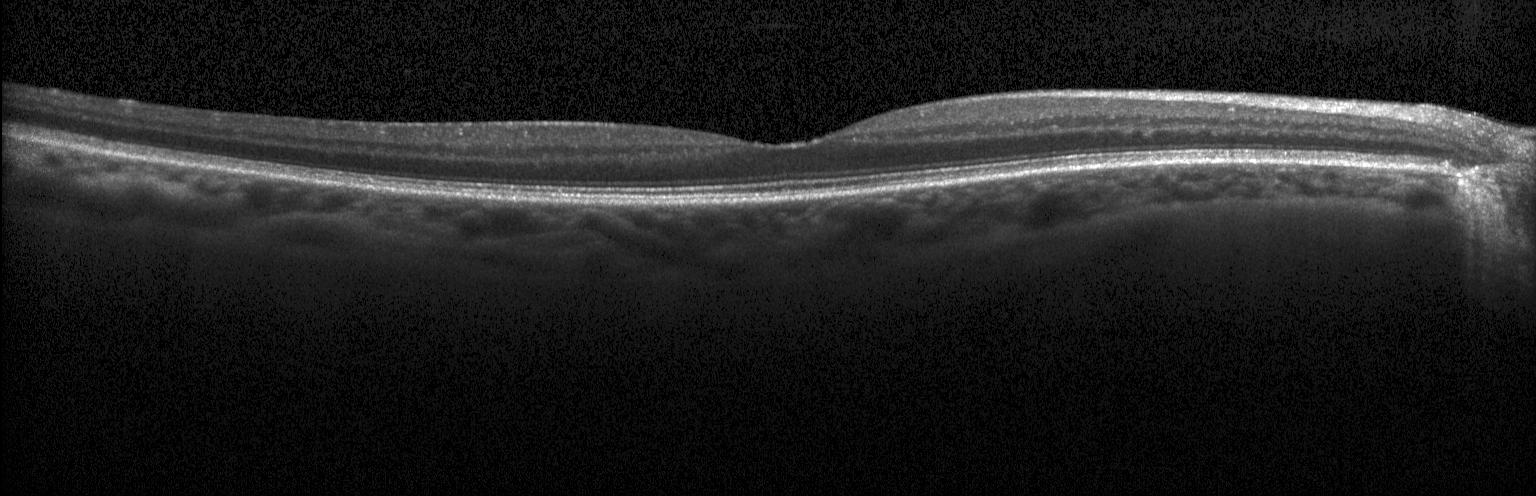 Retinal OCT cross-section showing no evidence of choroidal neovascularization, diabetic macular edema, or drusen.